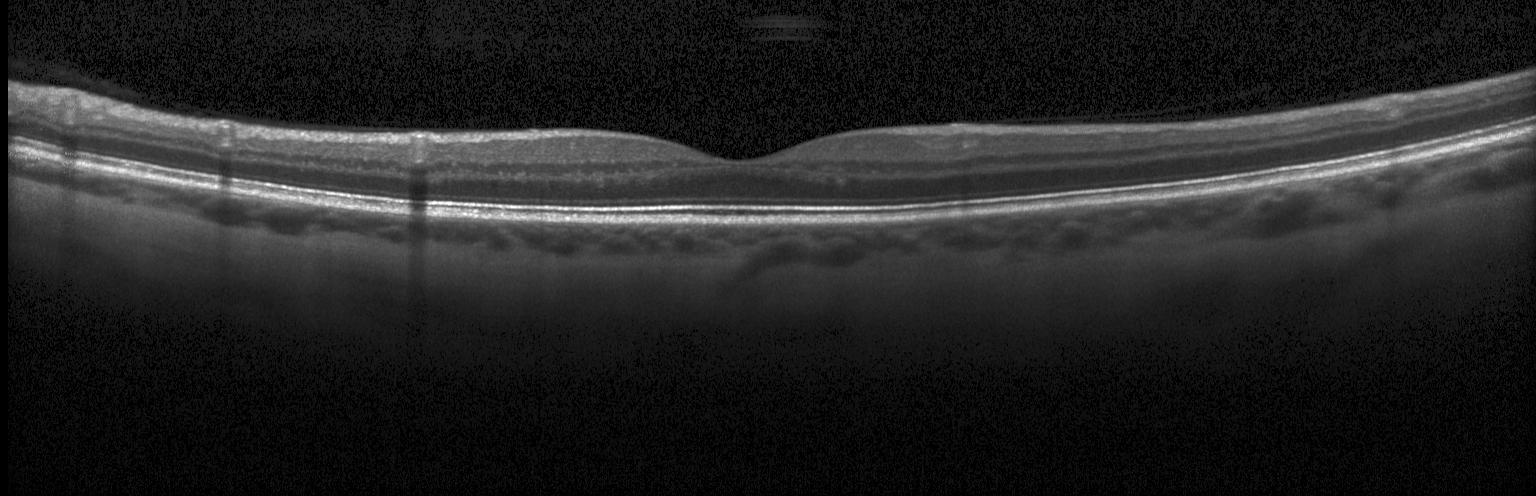

SD-OCT; fovea-centered; retinal OCT B-scan; Heidelberg Spectralis.
Neither choroidal neovascularization, diabetic macular edema, nor drusen.